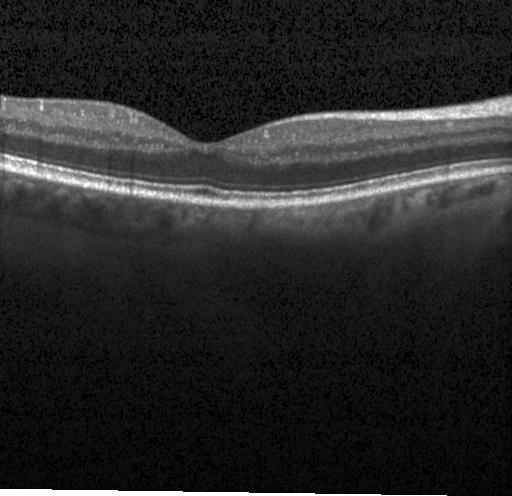
OCT line scan; Heidelberg Spectralis; macular scan — Dx: no evidence of choroidal neovascularization, diabetic macular edema, or drusen.